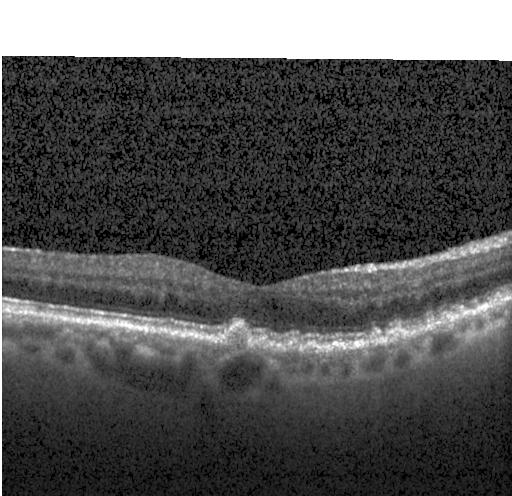 Optical coherence tomography B-scan.
Multiple drusen.